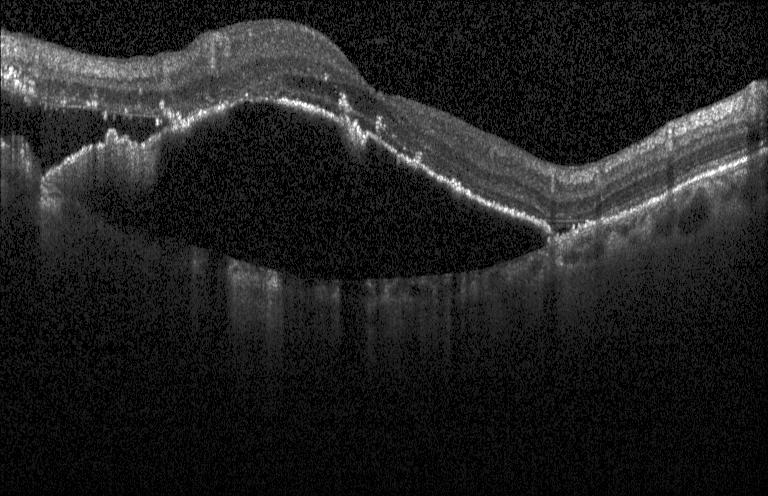

Spectral-domain OCT B-scan: a choroidal neovascular membrane.